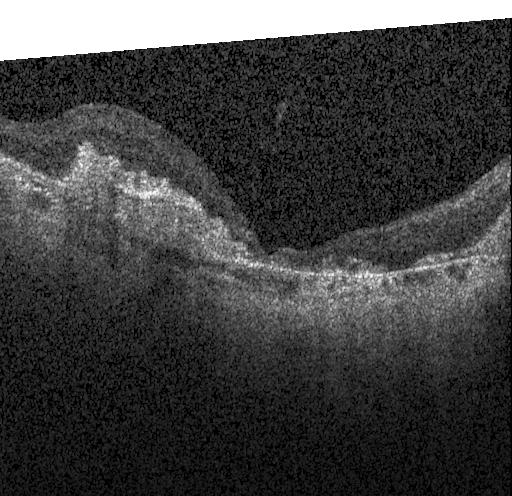

Centered on the fovea. Instrument: Heidelberg Spectralis. OCT line scan. Spectral-domain OCT.
Impression: a choroidal neovascular membrane.